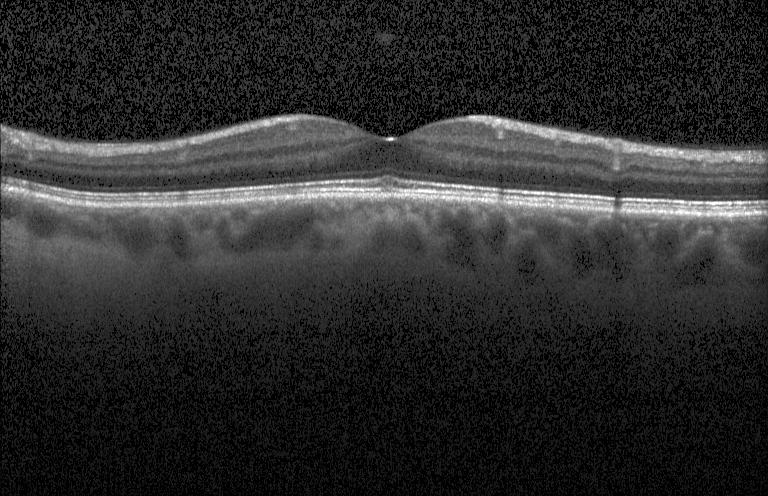
Impression: no CNV, no DME, and no drusen.